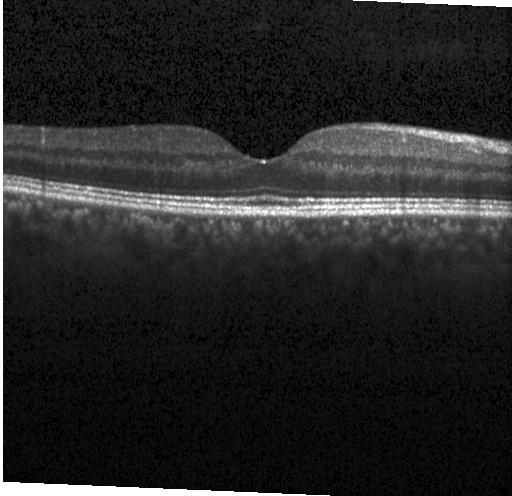
Impression: no choroidal neovascularization, no diabetic macular edema, and no drusen.